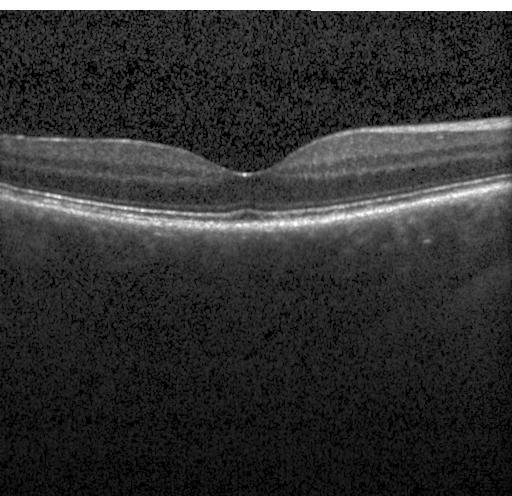
Spectral-domain optical coherence tomography. Optical coherence tomography scan. Centered on the fovea. Heidelberg Spectralis OCT system — OCT finding: no evidence of CNV, DME, or drusen.